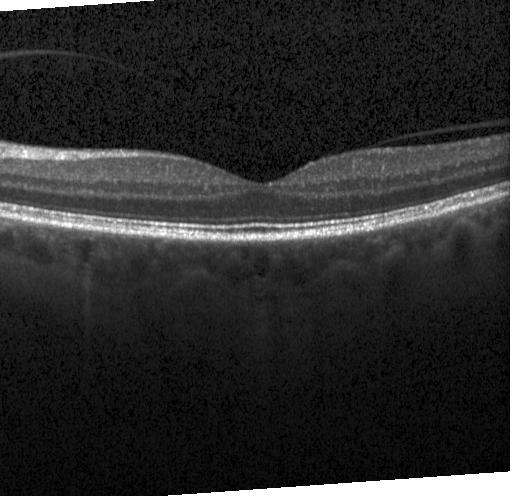 Fovea-centered, OCT B-scan.
This B-scan demonstrates no evidence of CNV, DME, or drusen.